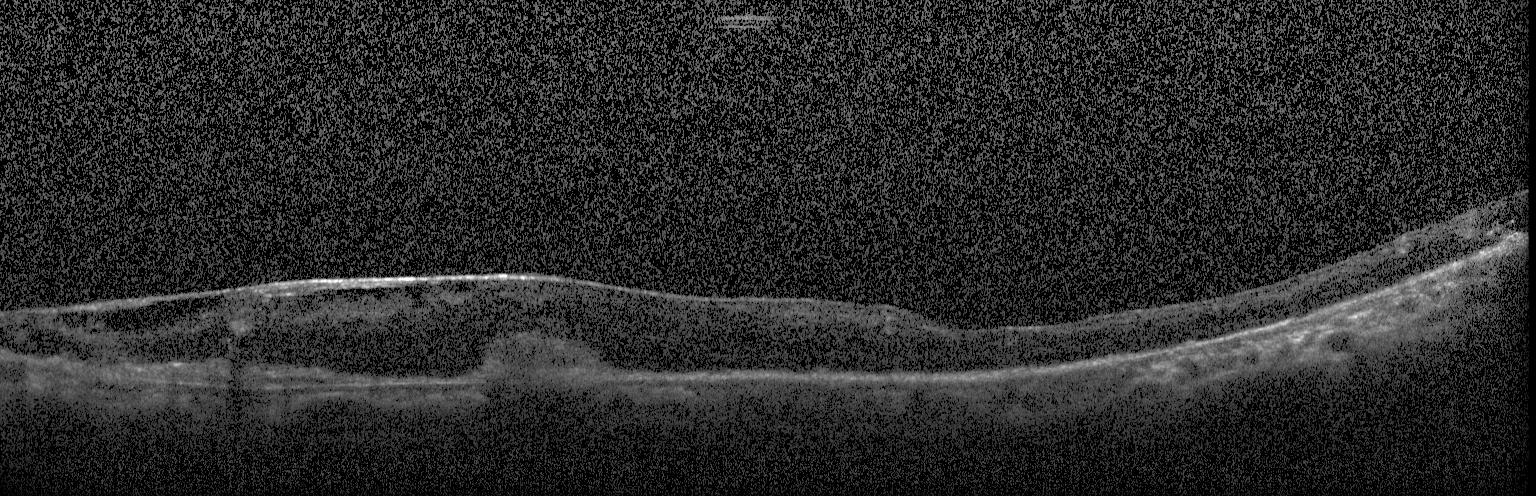

Diagnosis: a choroidal neovascular membrane.